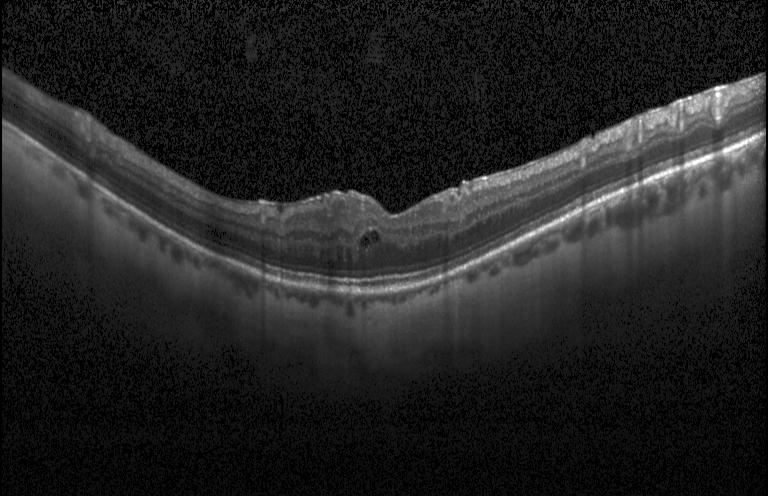
Finding: DME.